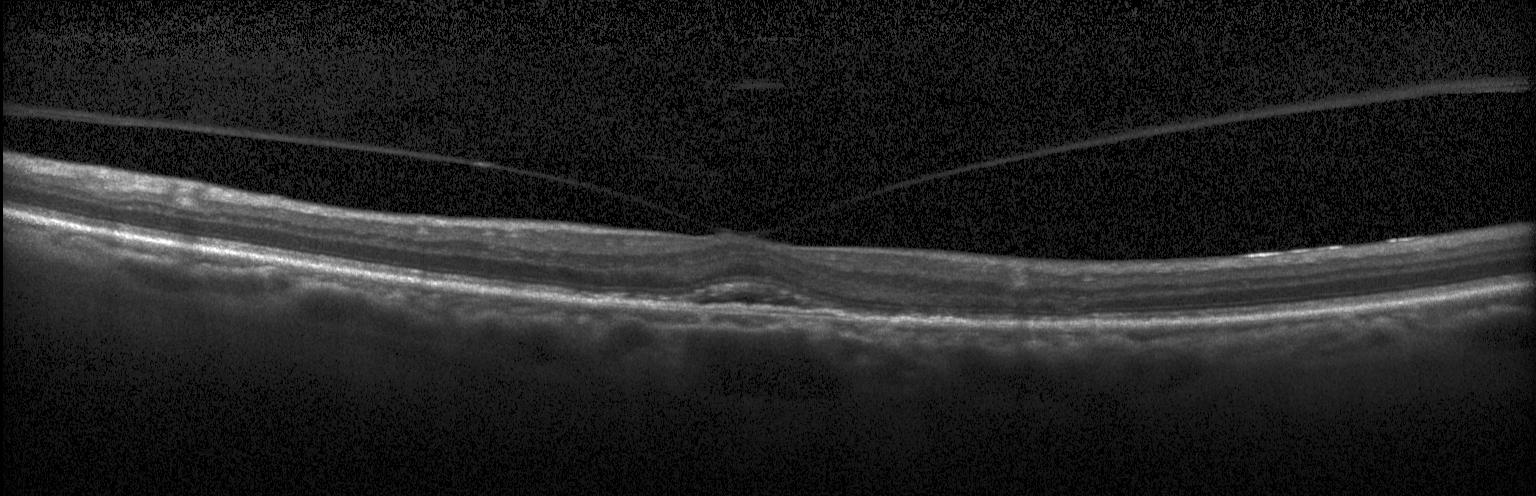 Retinal OCT cross-section showing choroidal neovascularization.